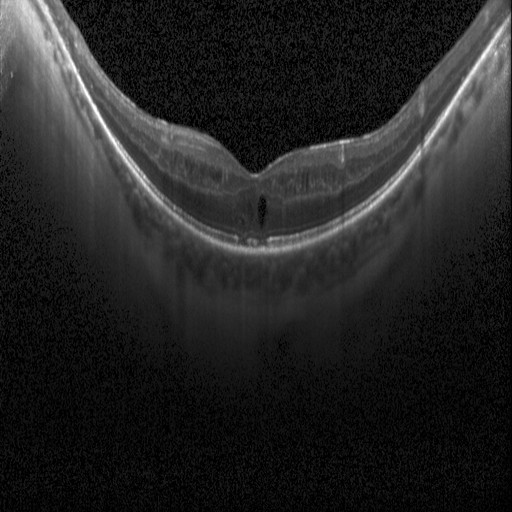 Dx: DME.